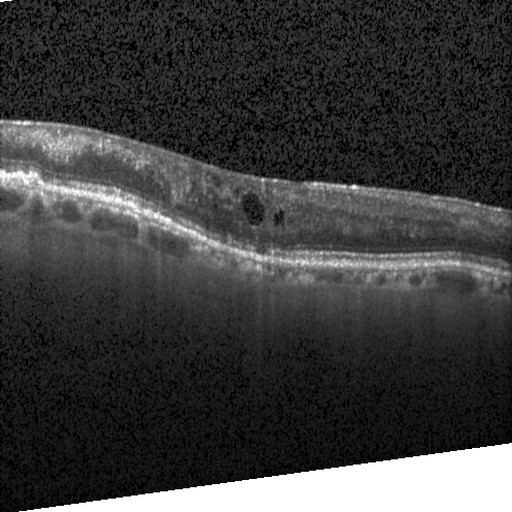 Centered on the fovea, Heidelberg Spectralis OCT system, optical coherence tomography B-scan.
Impression: diabetic macular edema (DME).